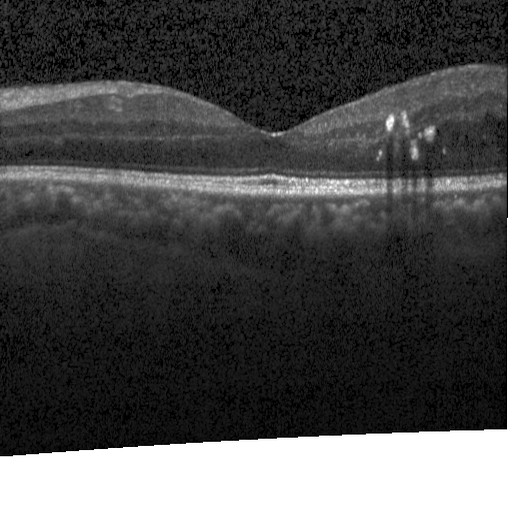 OCT scan showing diabetic macular edema (DME).